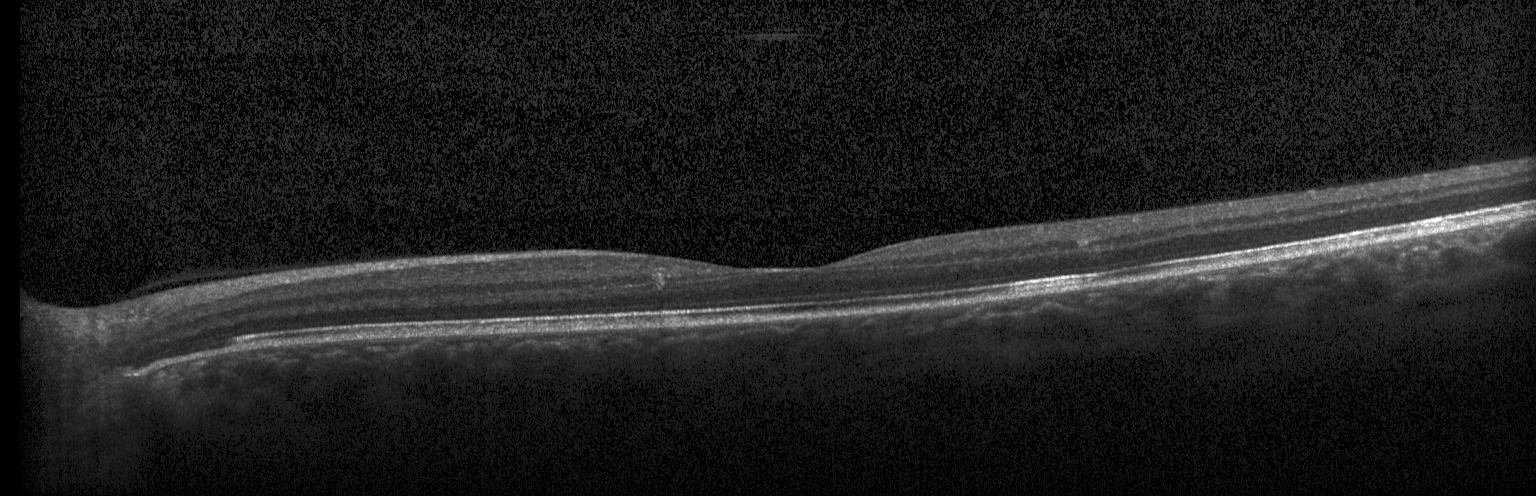
SD-OCT. Retinal OCT B-scan
Macular OCT: neither choroidal neovascularization, diabetic macular edema, nor drusen.